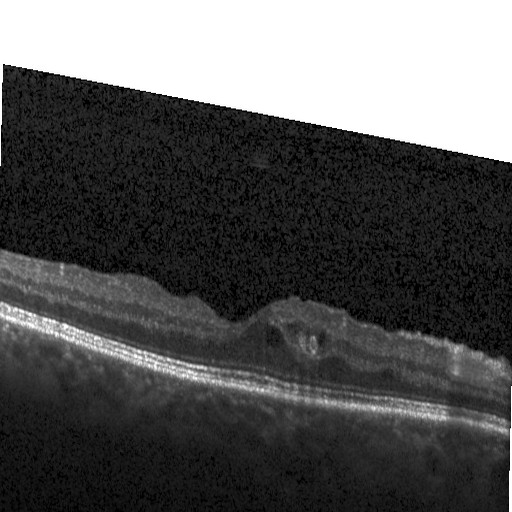
Diabetic macular edema (DME).